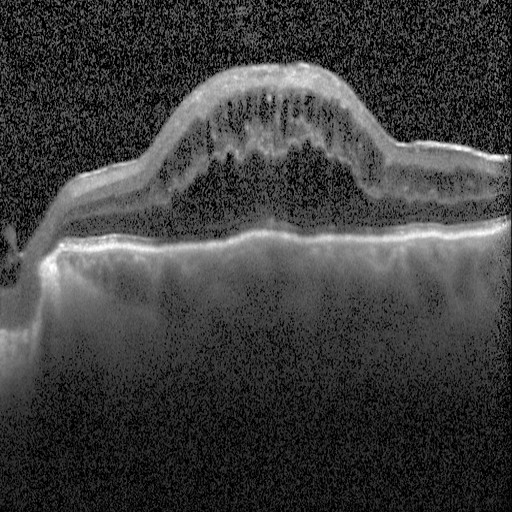
OCT line scan.
Finding: diabetic macular edema.